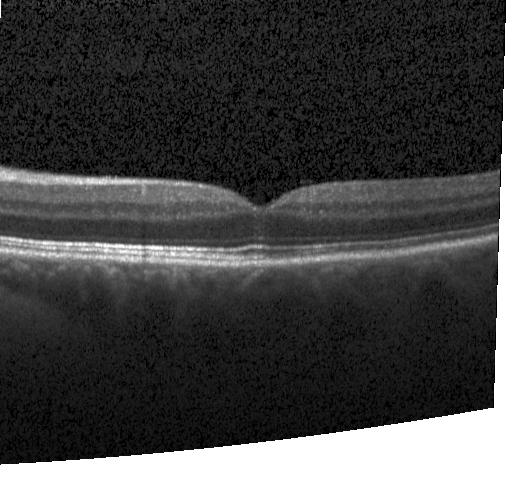
The scan shows no choroidal neovascularization, diabetic macular edema, or drusen.